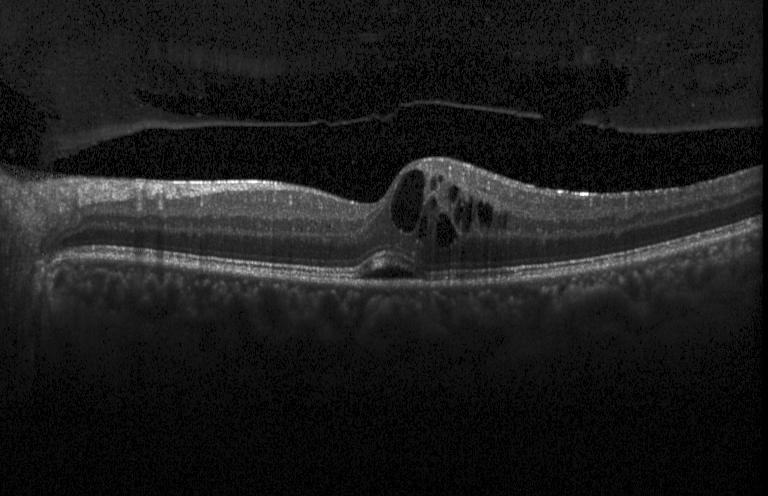 Impression: DME.